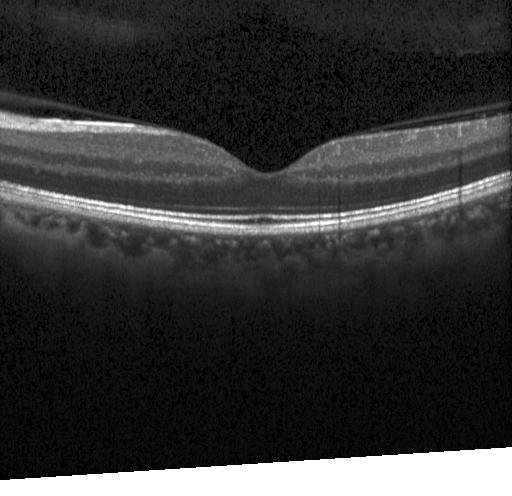

Fovea-centered; optical coherence tomography scan
Impression: neither CNV, DME, nor drusen.